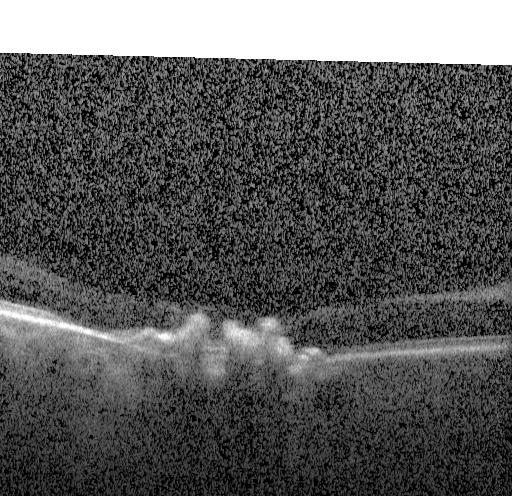

OCT B-scan — Impression: a choroidal neovascular membrane.